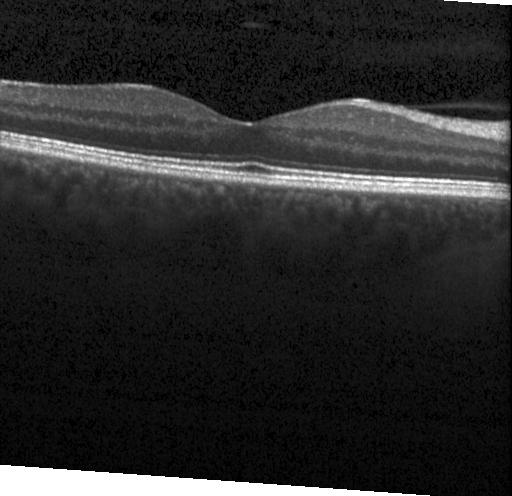

Impression: neither CNV, DME, nor drusen.